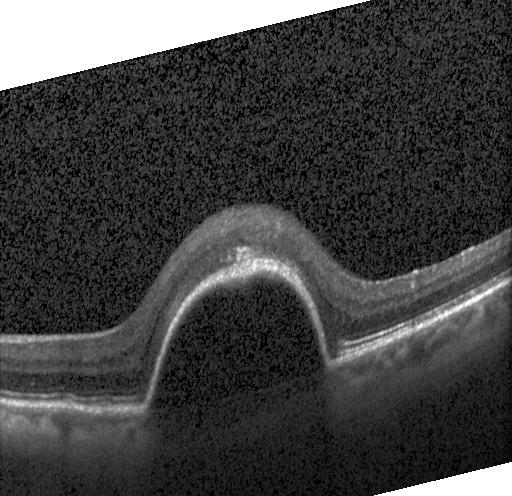

Acquired on a Heidelberg Spectralis, OCT line scan, spectral-domain OCT
Assessment: CNV.